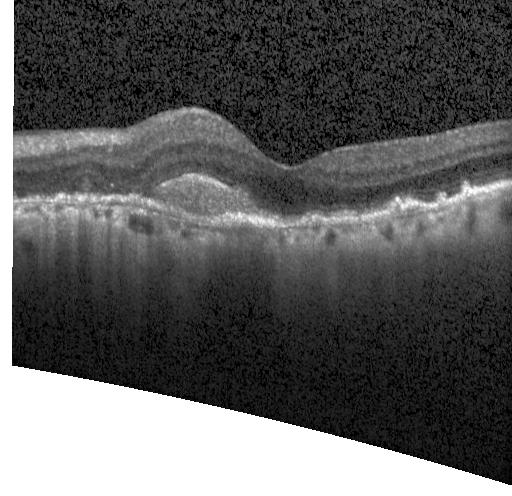
Acquired on a Heidelberg Spectralis; SD-OCT; OCT line scan.
Impression: a choroidal neovascular membrane.